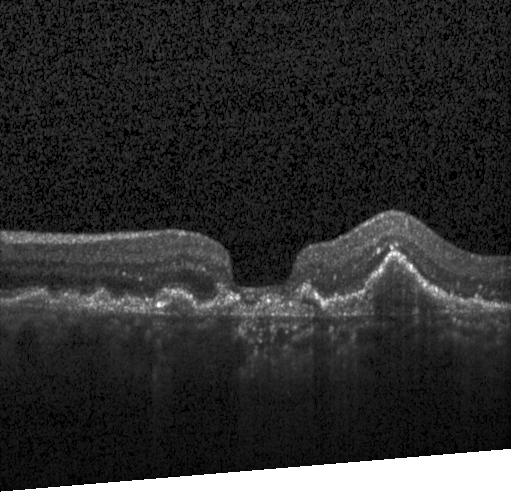
Heidelberg Spectralis · spectral-domain OCT · centered on the fovea · OCT line scan — Diagnosis: a choroidal neovascular membrane.